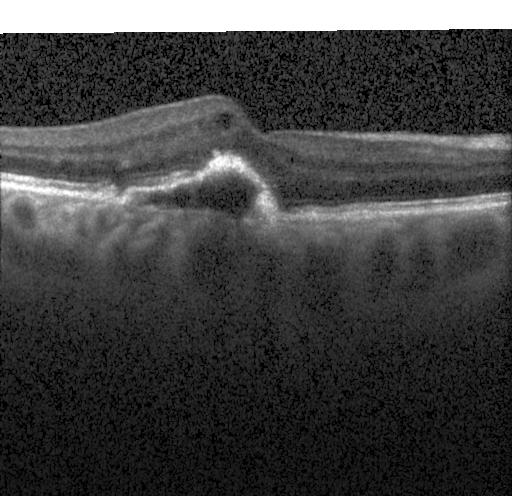

OCT B-scan; instrument: Heidelberg Spectralis
Finding: CNV.